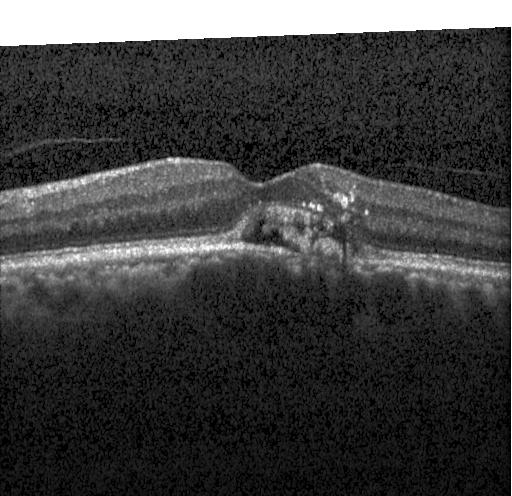 Retinal OCT cross-section. Impression: a choroidal neovascular membrane.